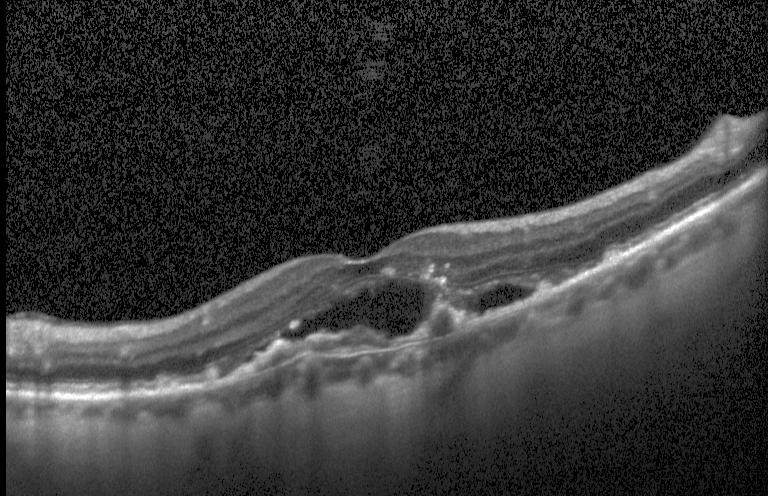
Retinal OCT cross-section · acquired on a Heidelberg Spectralis
Diagnosis: a choroidal neovascular membrane.